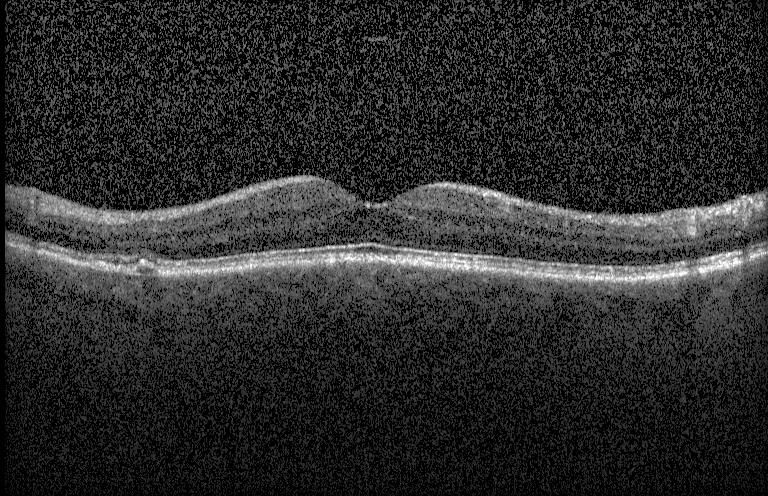
Horizontal scan through the fovea. Spectral-domain OCT. Retinal OCT B-scan
Macular OCT: a choroidal neovascular membrane.